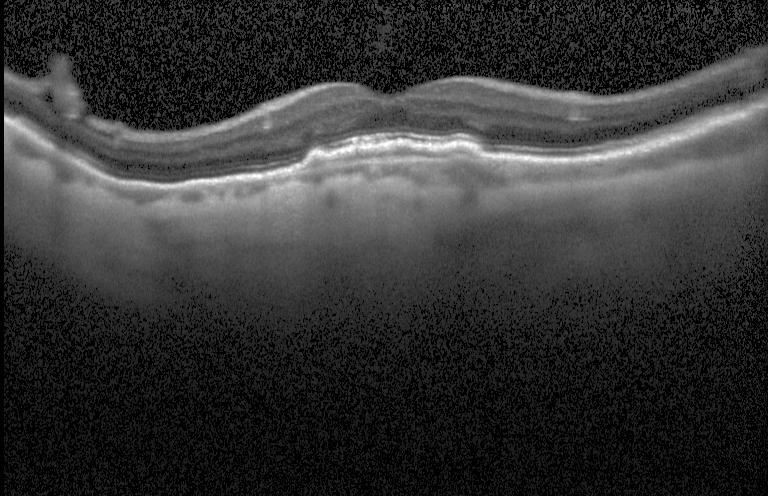
Spectral-domain optical coherence tomography; Heidelberg Spectralis; OCT line scan
This B-scan demonstrates a choroidal neovascular membrane.